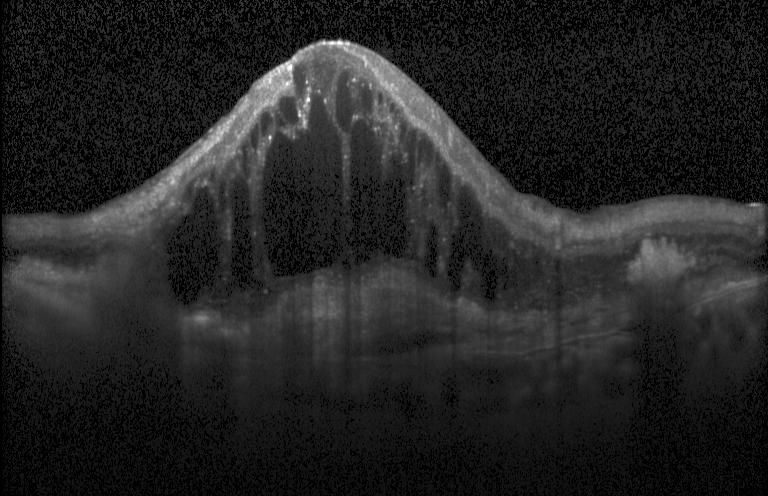

Retinal OCT cross-section. Impression: diabetic macular edema (DME).